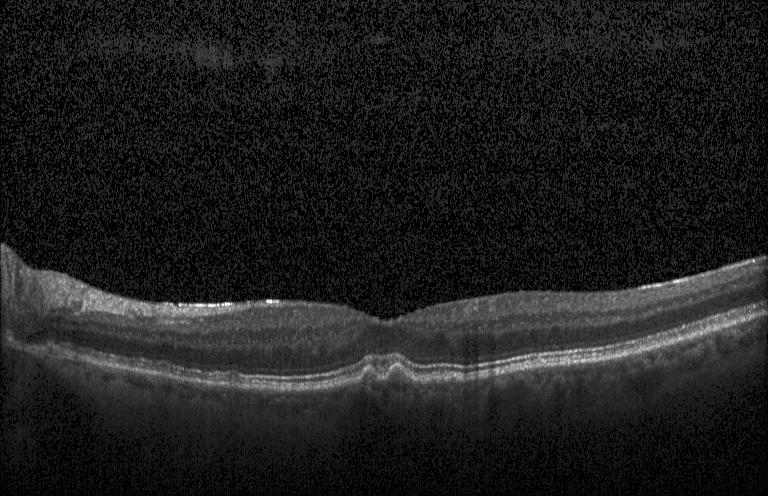

Impression: multiple drusen.